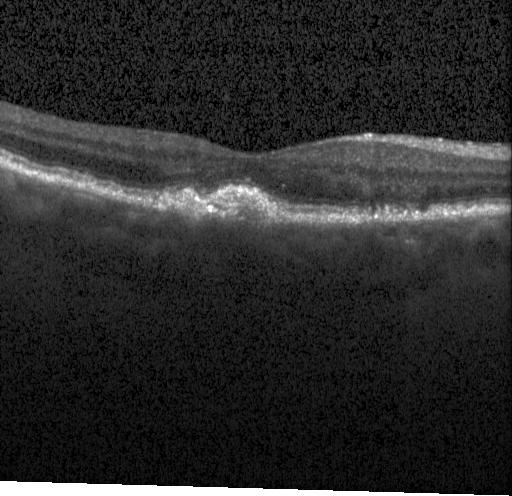
Macular OCT demonstrating a choroidal neovascular membrane.